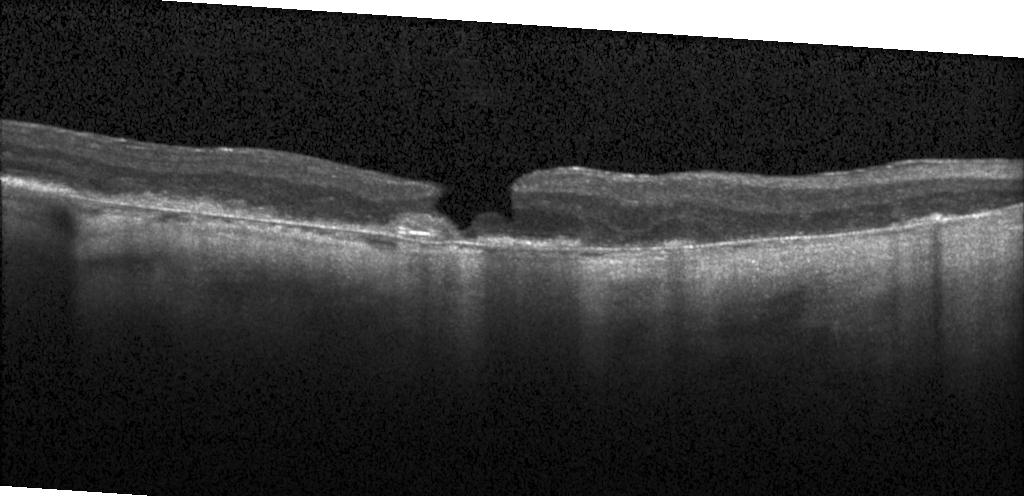 Diagnosis: a choroidal neovascular membrane.